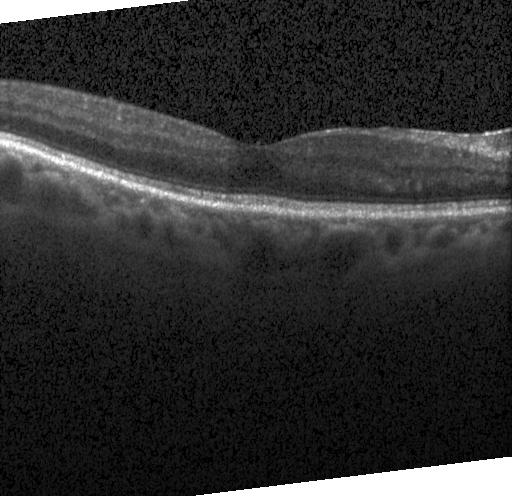

OCT finding: no CNV, DME, or drusen.